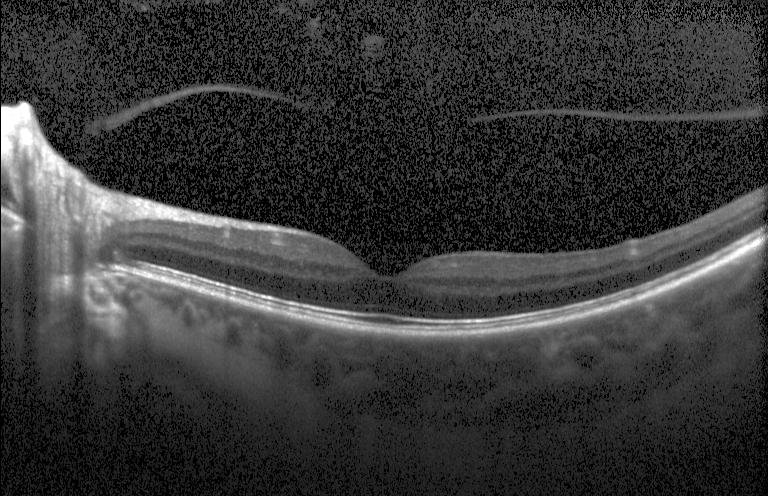 Optical coherence tomography B-scan, SD-OCT, acquired on a Heidelberg Spectralis
No choroidal neovascularization, diabetic macular edema, or drusen.